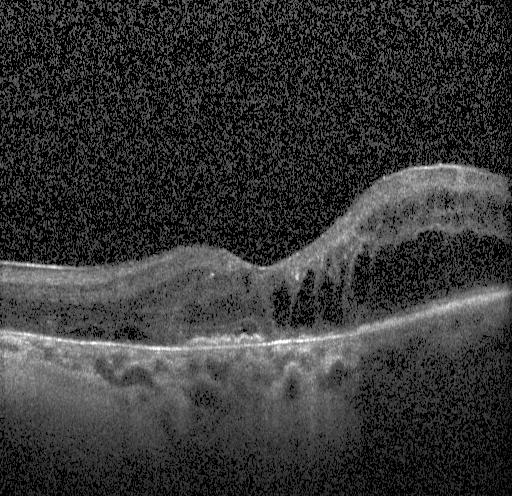
Fovea-centered · SD-OCT · instrument: Heidelberg Spectralis · OCT B-scan.
Diagnosis: a choroidal neovascular membrane.